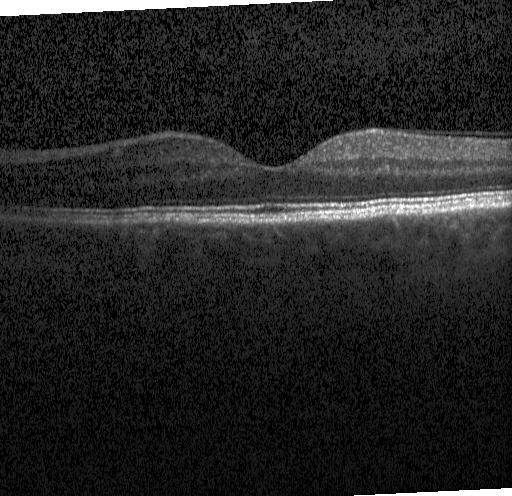
OCT finding: no choroidal neovascularization, no diabetic macular edema, and no drusen.